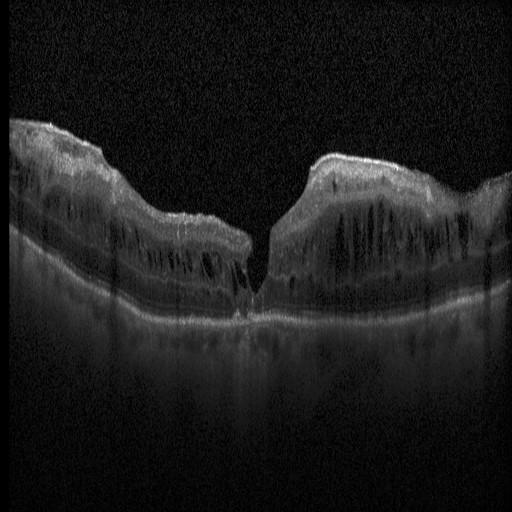
Spectral-domain OCT; Heidelberg Spectralis OCT system; through the macula; optical coherence tomography B-scan — Diagnosis: diabetic macular edema.